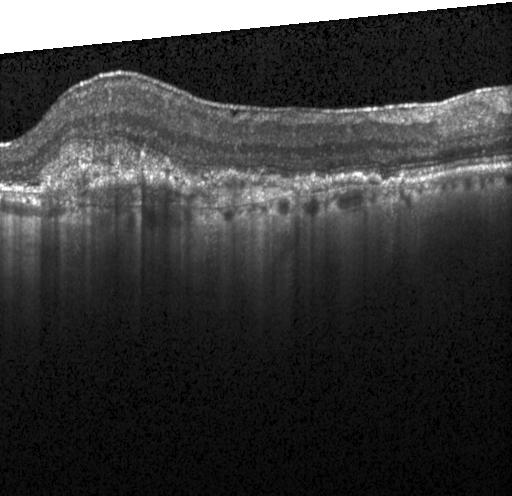
Macular OCT: a choroidal neovascular membrane.